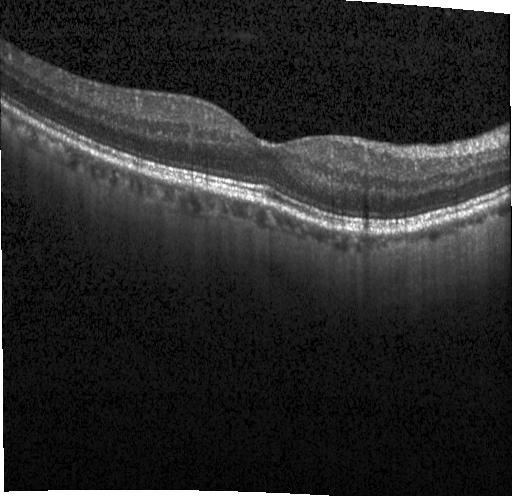
Optical coherence tomography B-scan. Heidelberg Spectralis. Through the macula.
The scan shows no evidence of choroidal neovascularization, diabetic macular edema, or drusen.